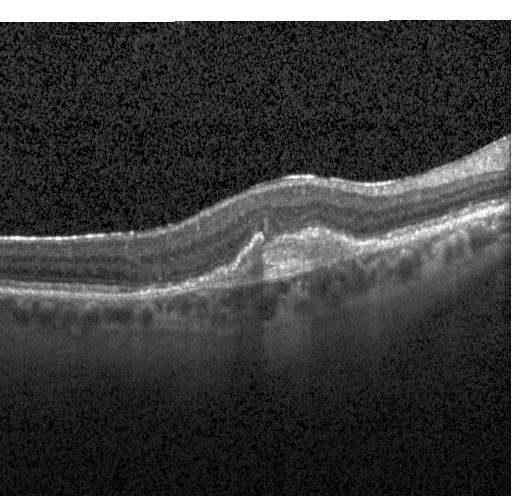

Macular OCT: choroidal neovascularization (CNV).